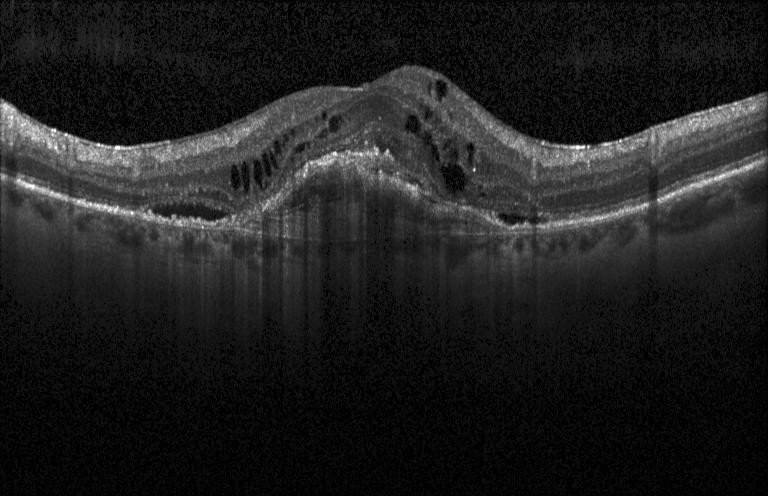 Spectral-domain optical coherence tomography · optical coherence tomography B-scan · Heidelberg Spectralis.
OCT finding: a choroidal neovascular membrane.